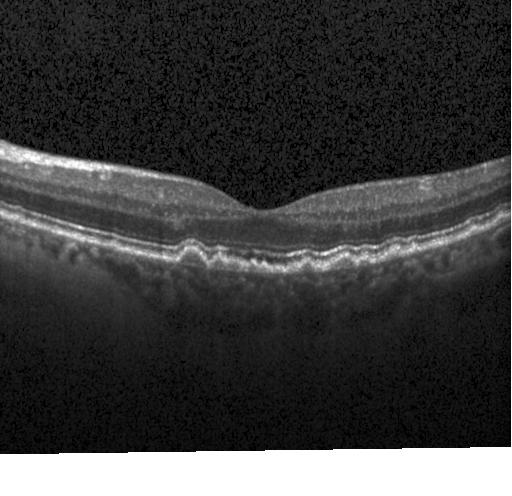

OCT line scan. Diagnosis: sub-RPE drusenoid deposits.